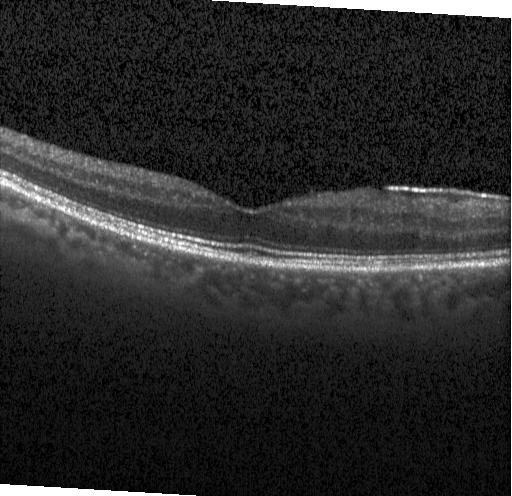 Diagnosis: no evidence of choroidal neovascularization, diabetic macular edema, or drusen.